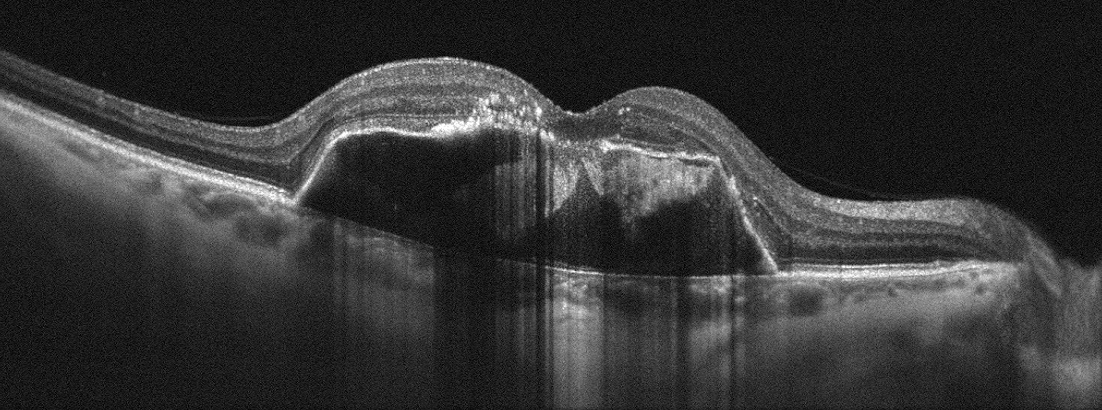
Retinal OCT cross-section
Impression: age-related macular degeneration.